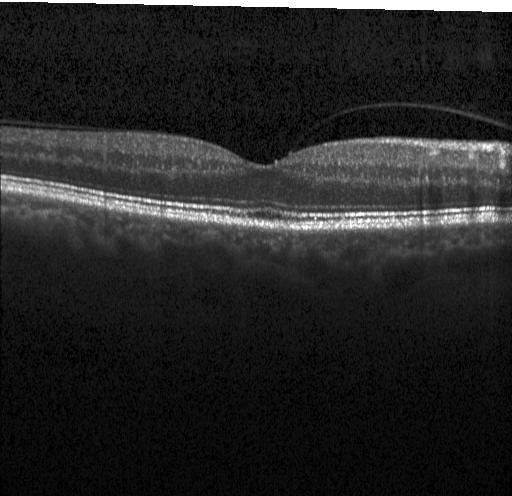 OCT line scan, Heidelberg Spectralis OCT system, spectral-domain optical coherence tomography. Finding: no choroidal neovascularization, diabetic macular edema, or drusen.